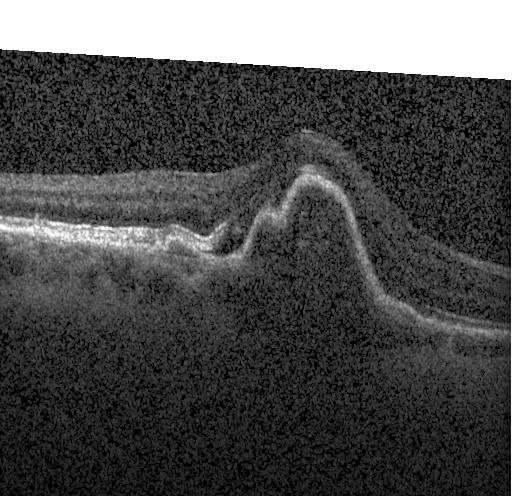
Spectral-domain optical coherence tomography, macular scan, Heidelberg Spectralis, OCT line scan.
Finding: a choroidal neovascular membrane.